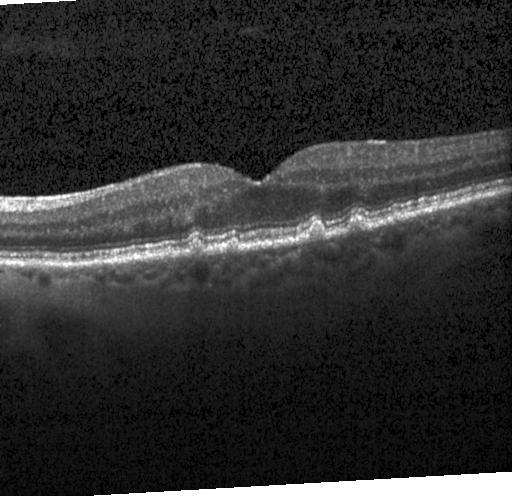 Heidelberg Spectralis · horizontal scan through the fovea · optical coherence tomography B-scan · SD-OCT
Impression: drusen.